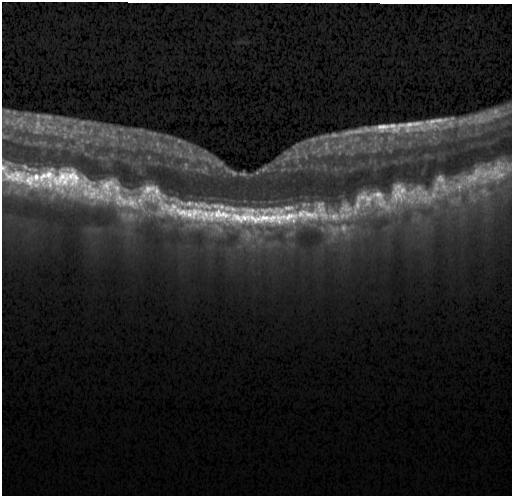

Spectral-domain optical coherence tomography. Retinal OCT cross-section
Dx: sub-RPE drusenoid deposits.